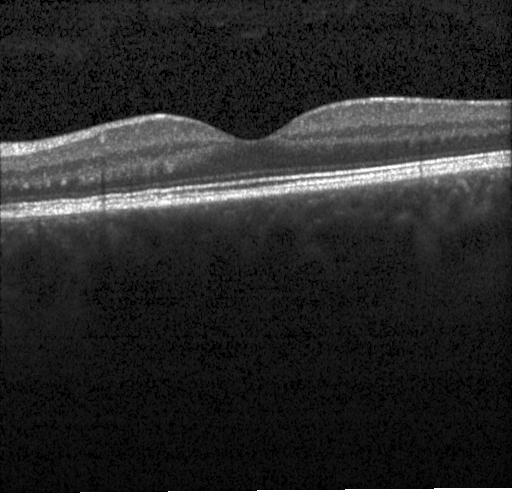

Spectral-domain optical coherence tomography; optical coherence tomography B-scan; horizontal scan through the fovea
Macular OCT: neither CNV, DME, nor drusen.